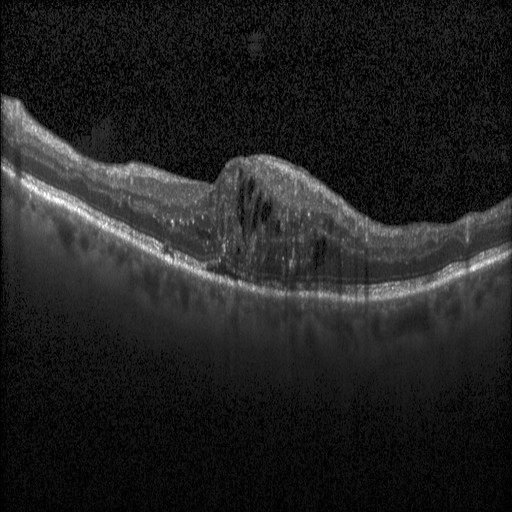 This B-scan demonstrates DME.